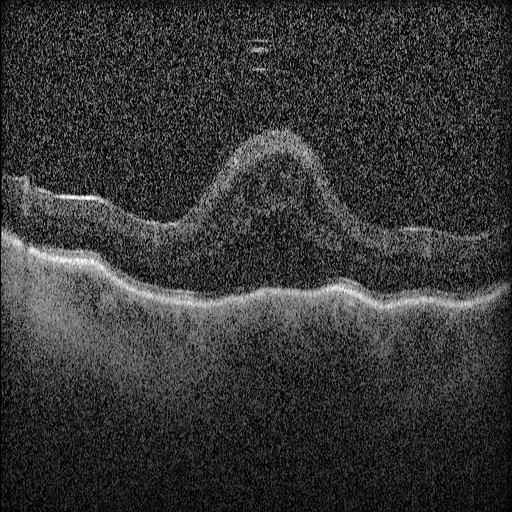

Macular OCT: DME.